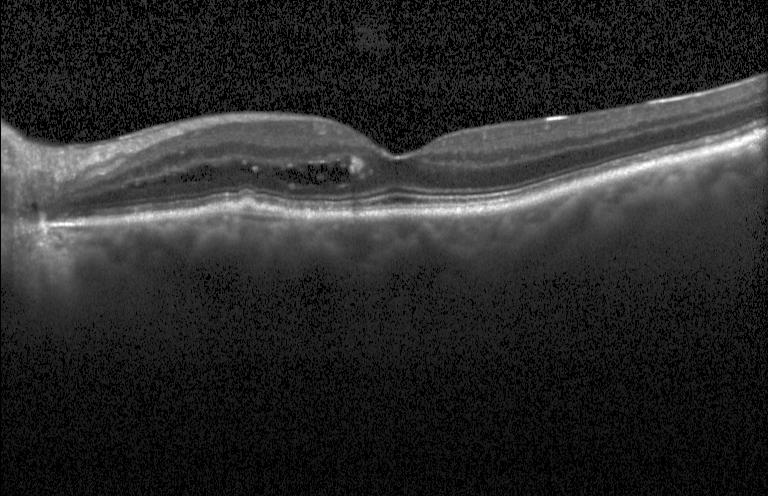
Macular OCT demonstrating DME.